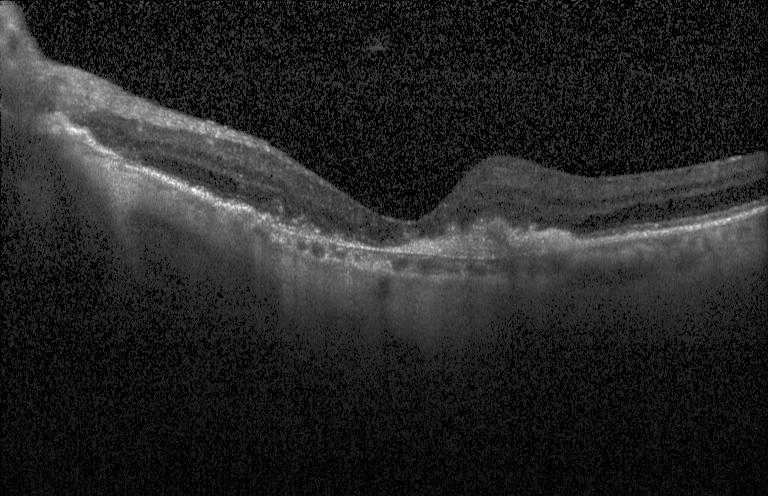 Assessment: choroidal neovascularization.